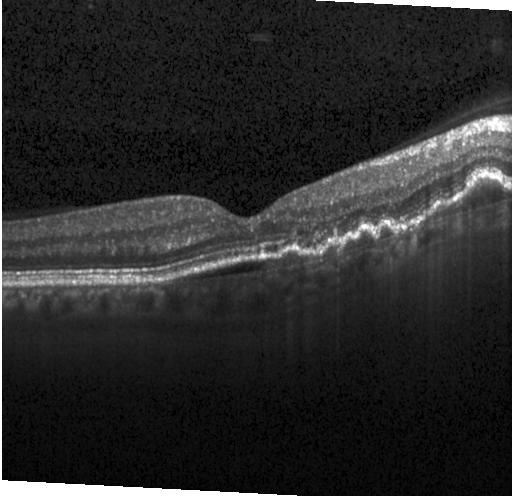

OCT finding: a choroidal neovascular membrane.